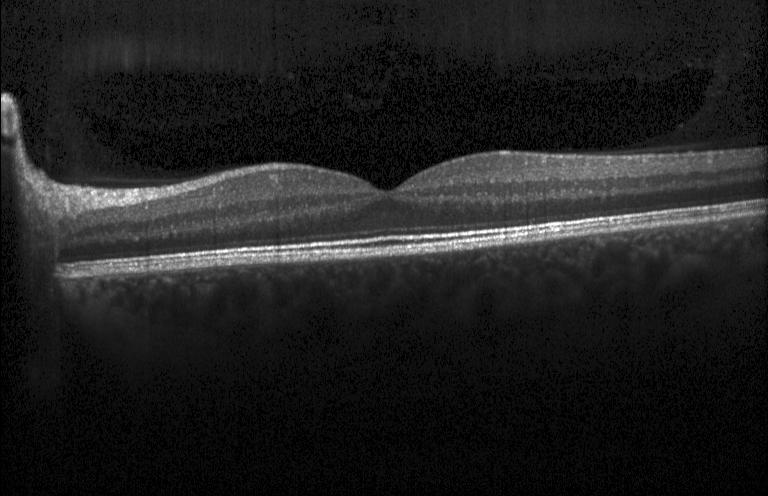

Through the macula. Spectral-domain optical coherence tomography. Optical coherence tomography B-scan. Assessment: neither choroidal neovascularization, diabetic macular edema, nor drusen.